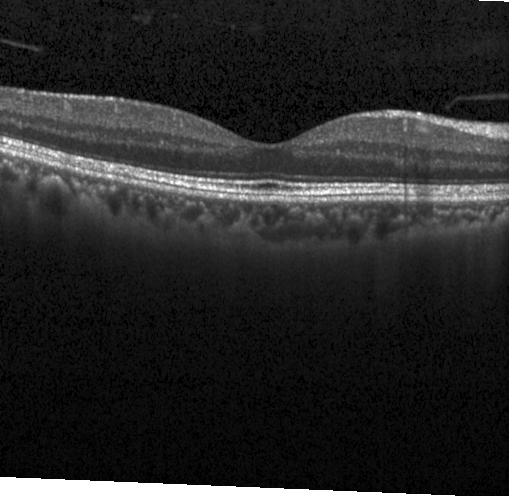

No choroidal neovascularization, no diabetic macular edema, and no drusen.